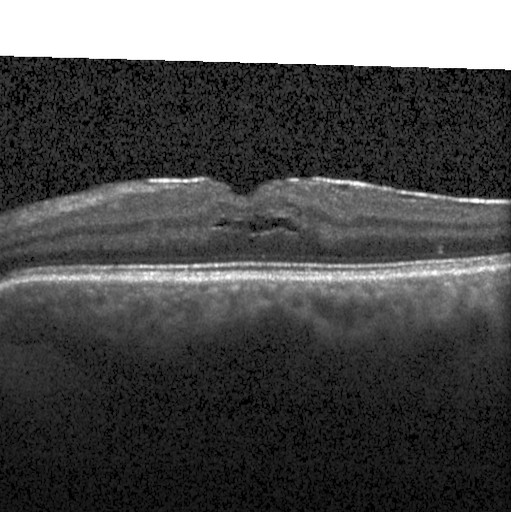

Retinal OCT cross-section
Diagnosis: diabetic macular edema.